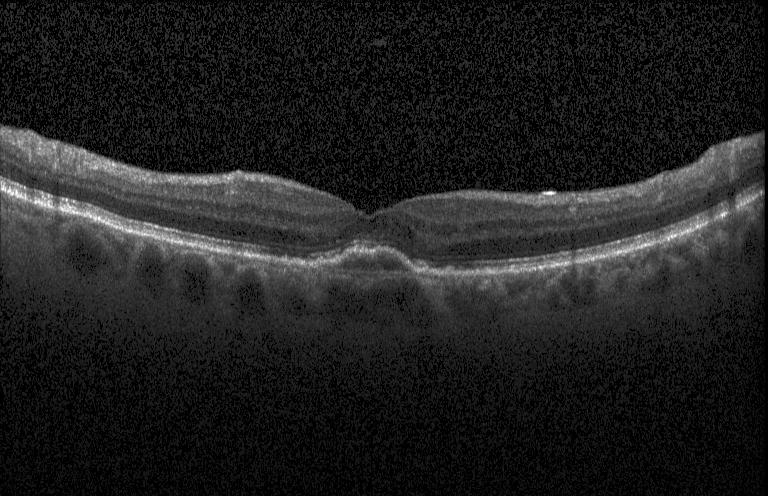 Diagnosis: a choroidal neovascular membrane.